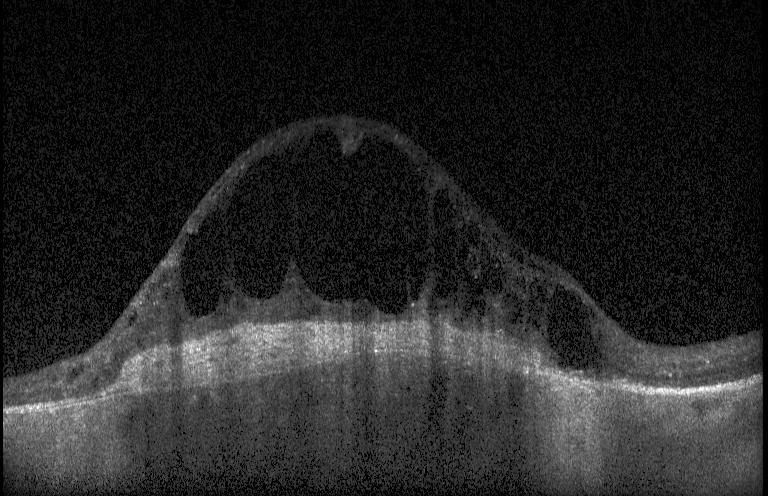

Retinal OCT cross-section.
Diagnosis: choroidal neovascularization (CNV).